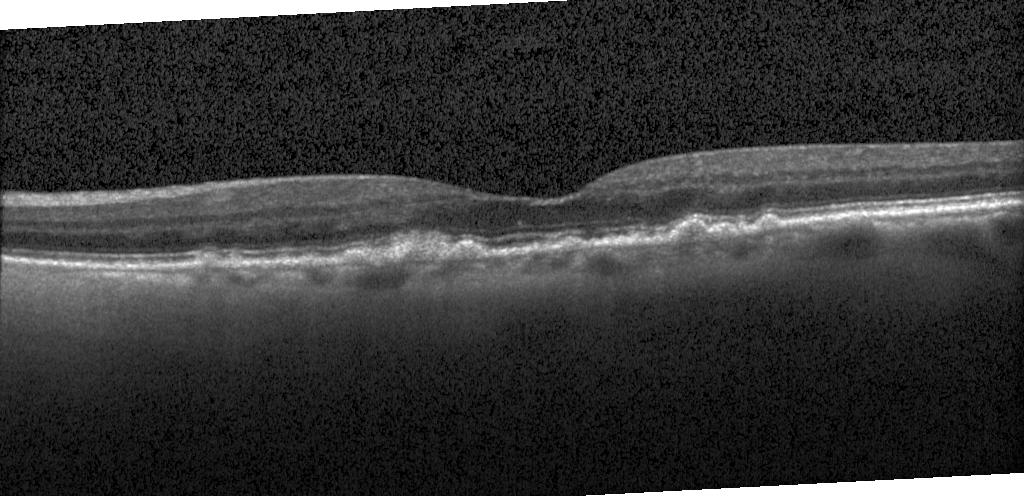

Assessment: sub-RPE drusenoid deposits.